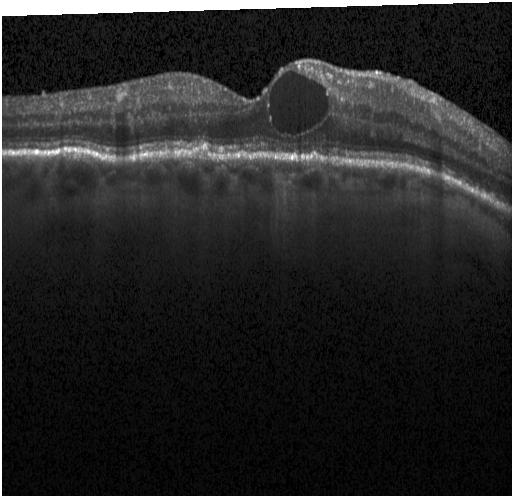
Acquired on a Heidelberg Spectralis. SD-OCT. Optical coherence tomography scan
Finding: a choroidal neovascular membrane.